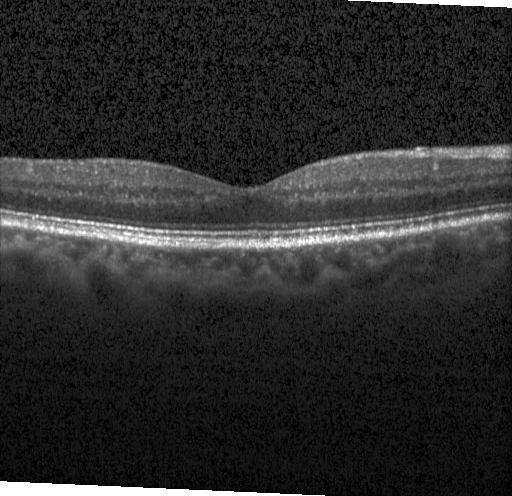
OCT line scan; spectral-domain optical coherence tomography.
Assessment: neither CNV, DME, nor drusen.